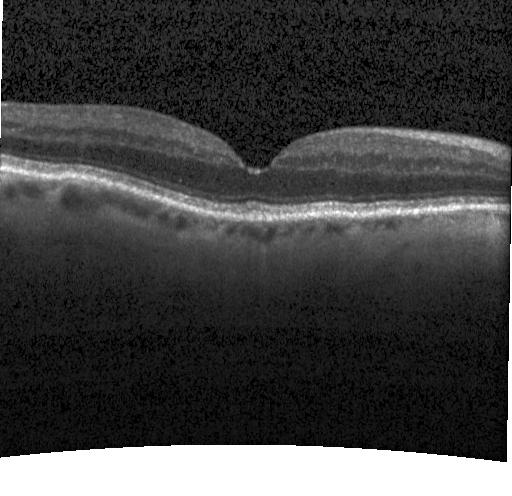
This B-scan demonstrates no evidence of choroidal neovascularization, diabetic macular edema, or drusen.